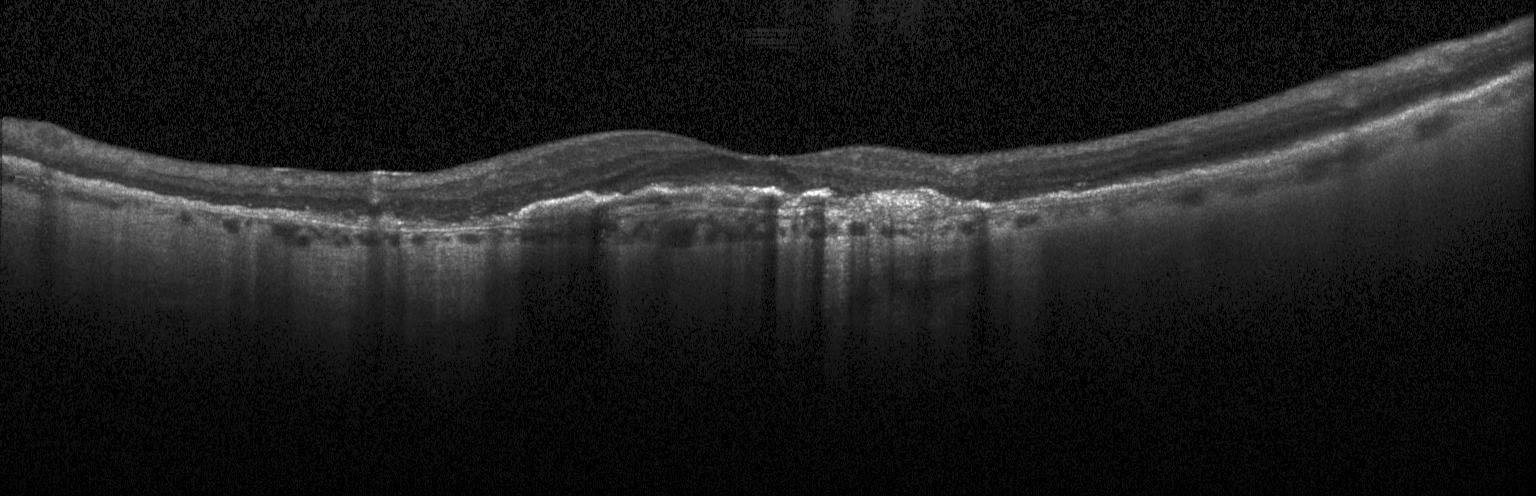
Finding: a choroidal neovascular membrane.